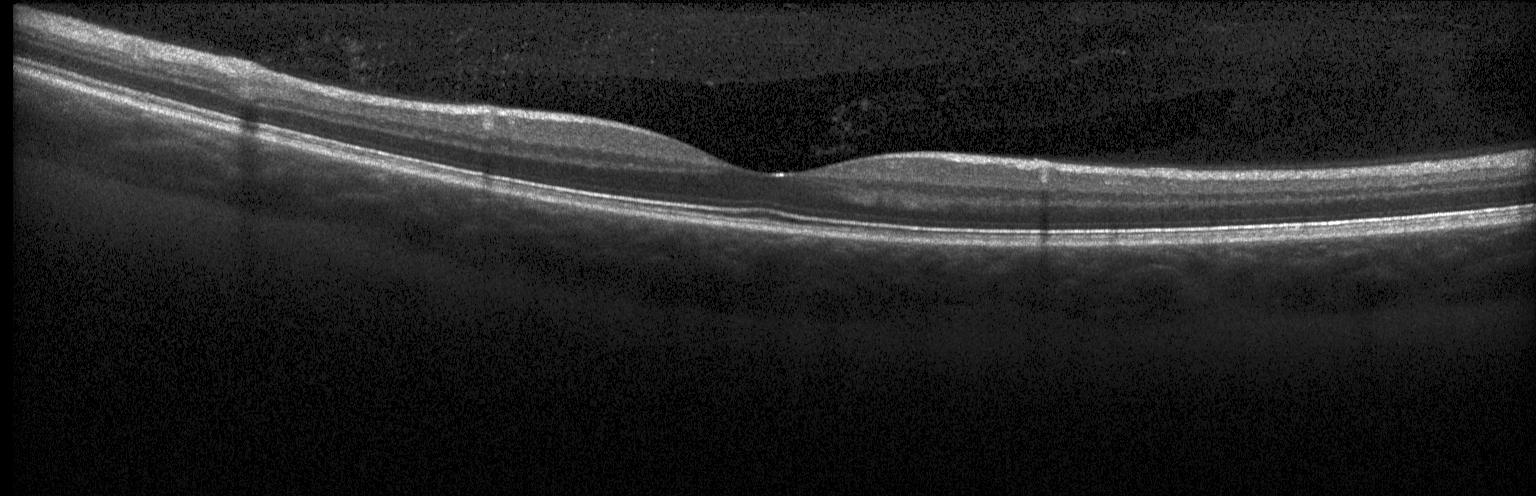 Diagnosis: no choroidal neovascularization, no diabetic macular edema, and no drusen.